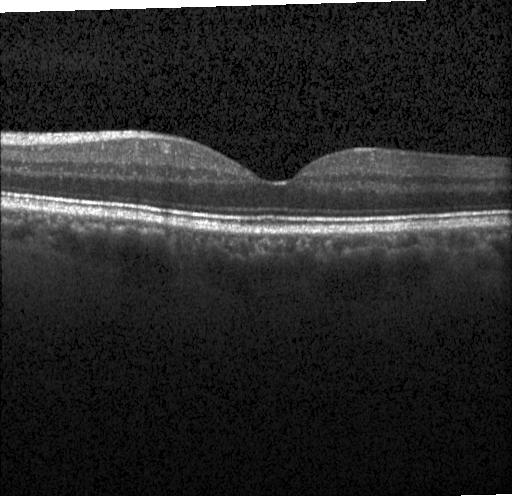 Spectral-domain OCT B-scan: no choroidal neovascularization, diabetic macular edema, or drusen.